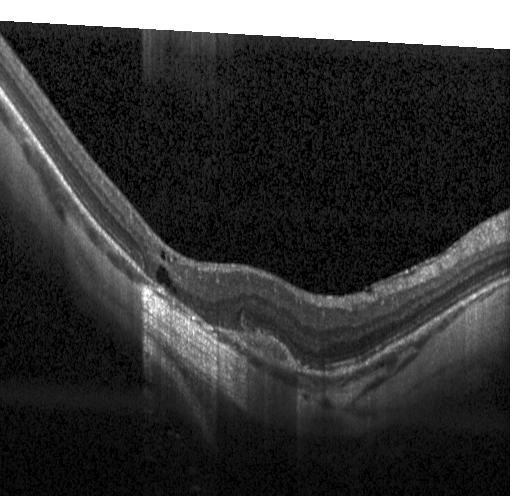

Optical coherence tomography B-scan · fovea-centered
This B-scan demonstrates CNV.